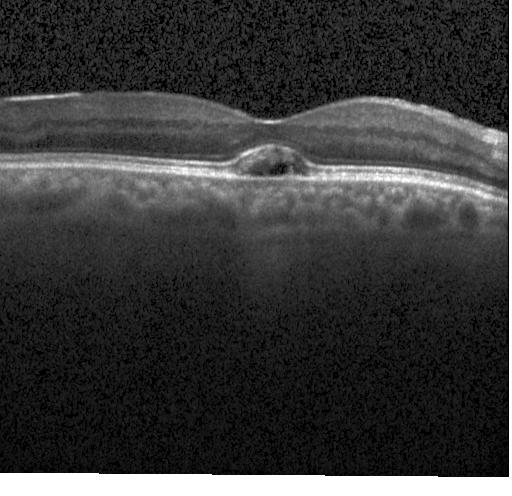
Dx: a choroidal neovascular membrane.